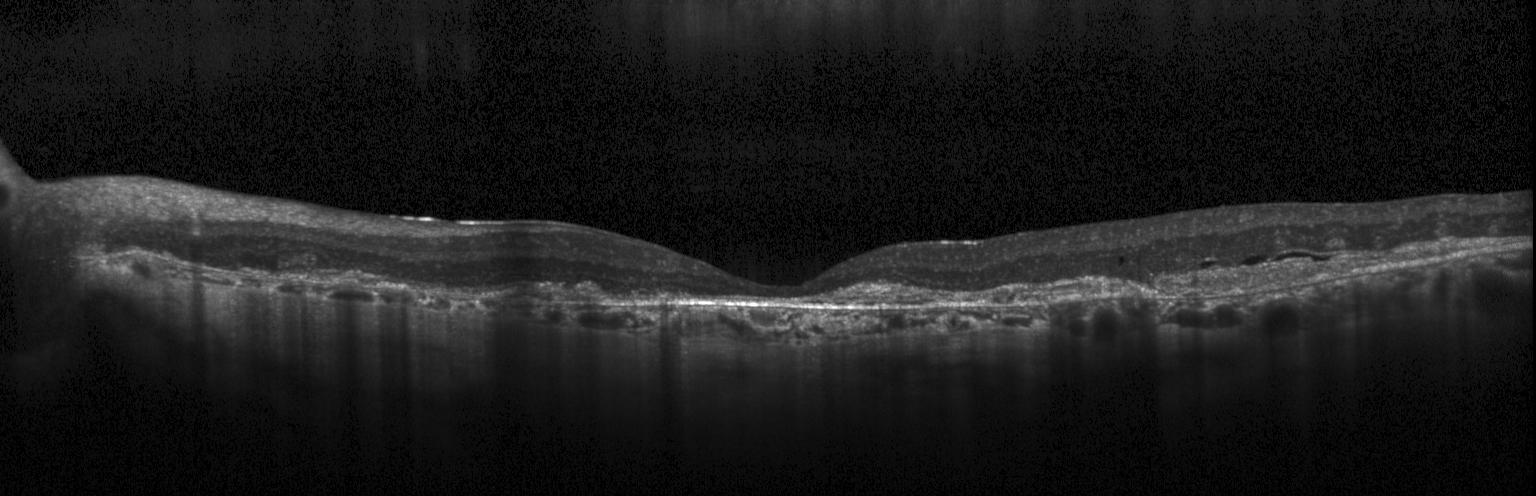
Retinal OCT B-scan
Diagnosis: choroidal neovascularization.